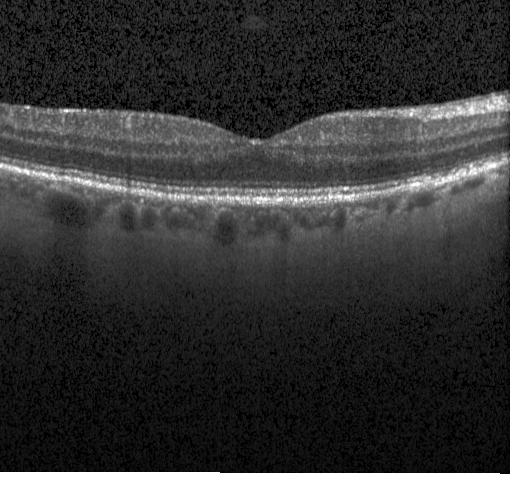 Instrument: Heidelberg Spectralis · through the macula · retinal OCT B-scan · SD-OCT. Impression: no choroidal neovascularization, no diabetic macular edema, and no drusen.